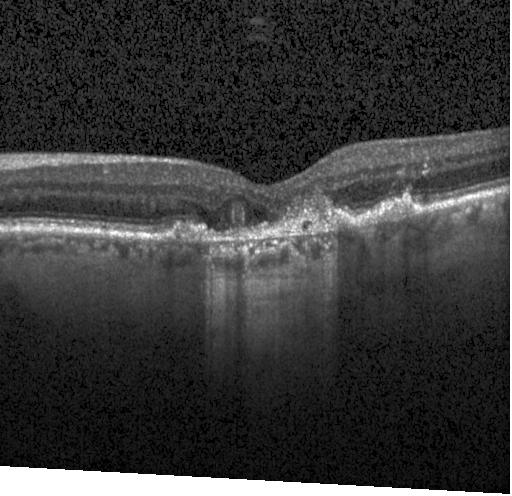

Macular OCT: a choroidal neovascular membrane.